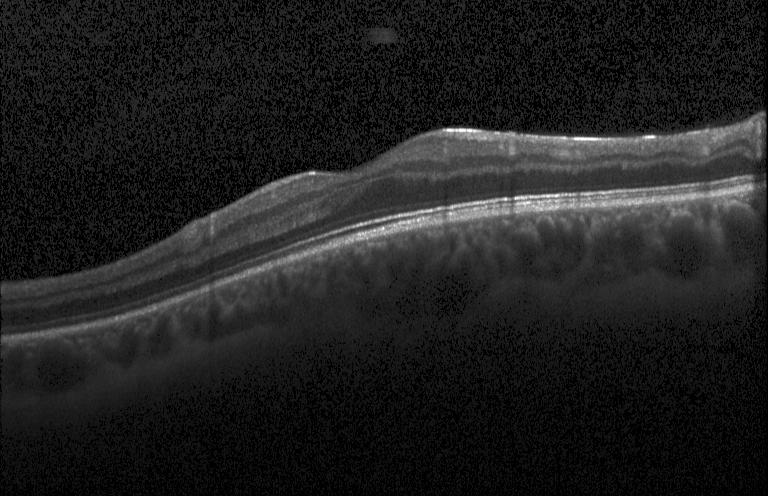 This B-scan demonstrates no evidence of choroidal neovascularization, diabetic macular edema, or drusen.